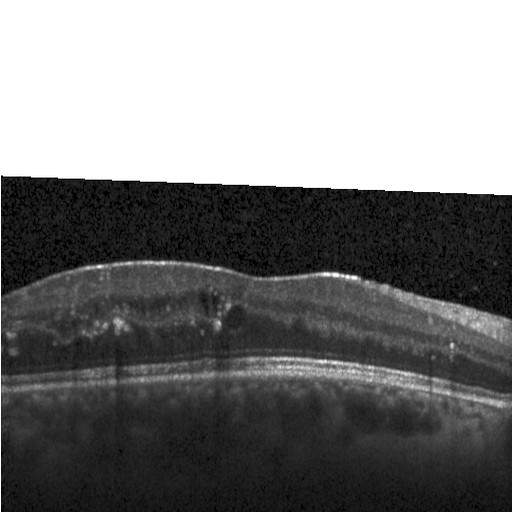

Optical coherence tomography B-scan, through the macula.
Diagnosis: diabetic macular edema.